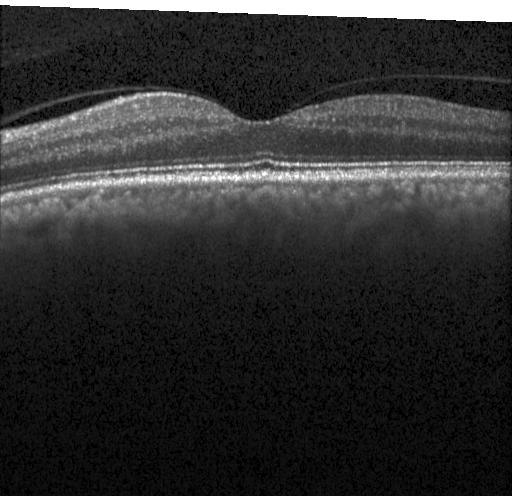

Acquired on a Heidelberg Spectralis; retinal OCT cross-section. This B-scan demonstrates no choroidal neovascularization, no diabetic macular edema, and no drusen.